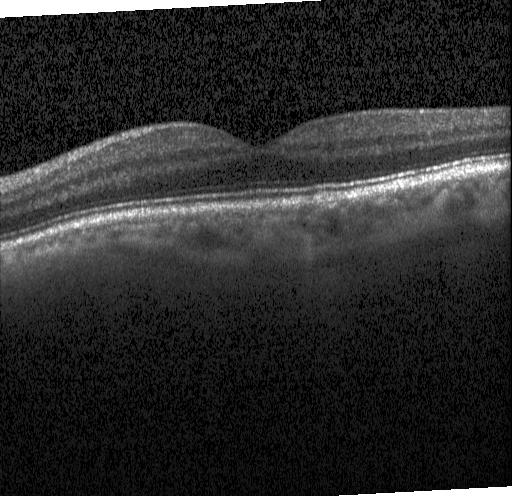
Optical coherence tomography scan — Impression: no choroidal neovascularization, no diabetic macular edema, and no drusen.